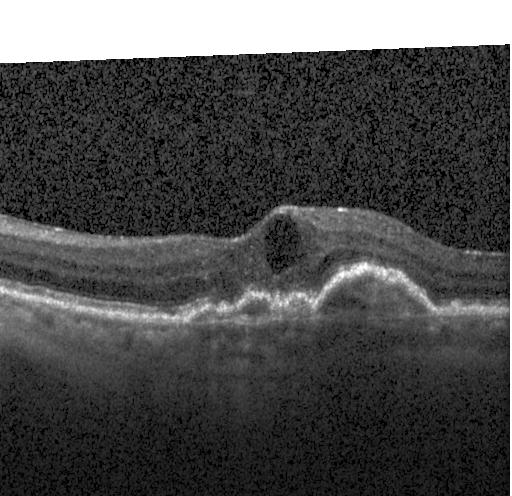
Optical coherence tomography scan
Diagnosis: choroidal neovascularization (CNV).